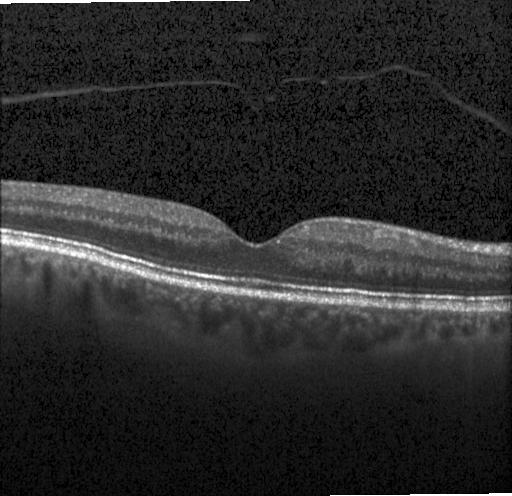
OCT B-scan. Impression: no choroidal neovascularization, no diabetic macular edema, and no drusen.